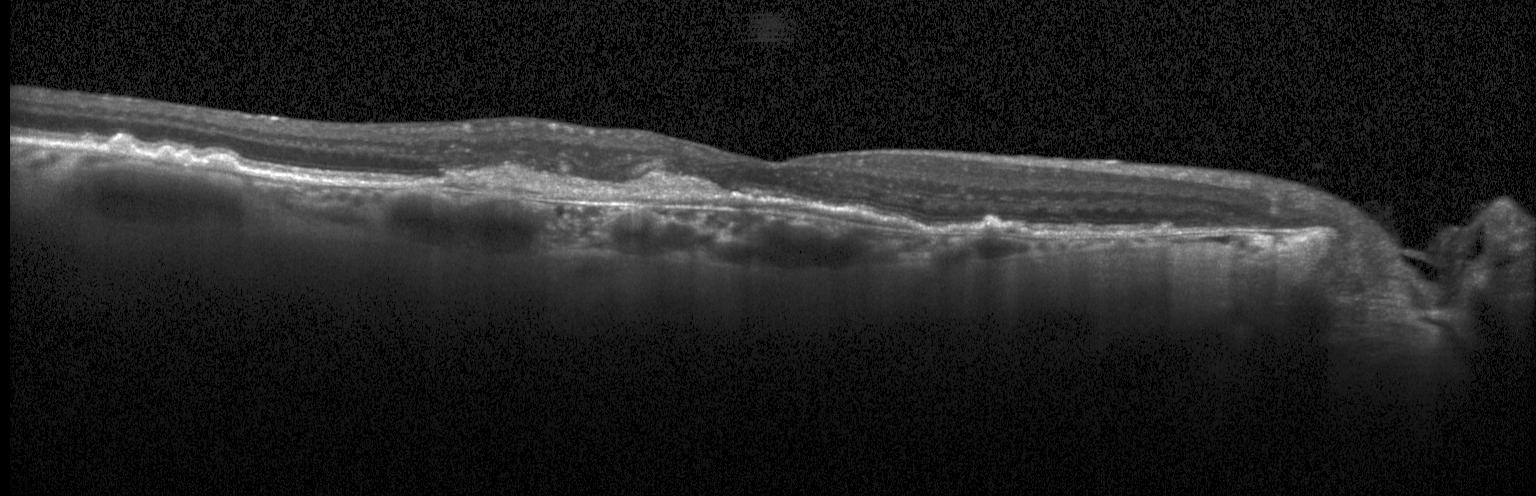

Macular OCT demonstrating a choroidal neovascular membrane.